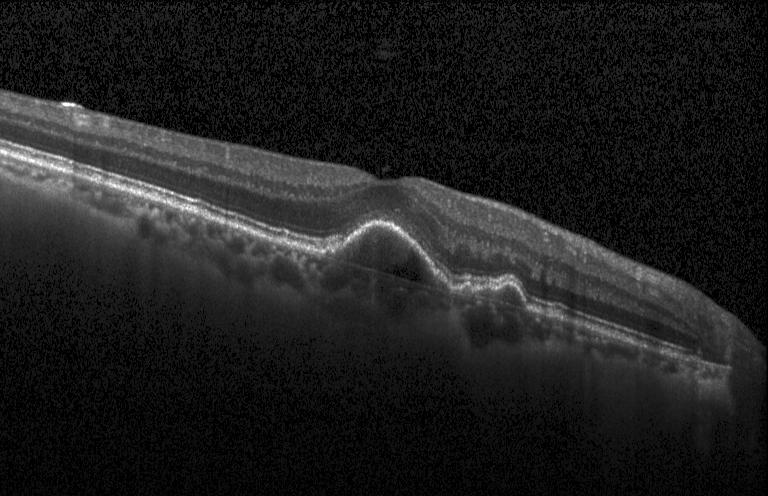

Spectral-domain optical coherence tomography, retinal OCT B-scan, centered on the fovea — This B-scan demonstrates choroidal neovascularization (CNV).